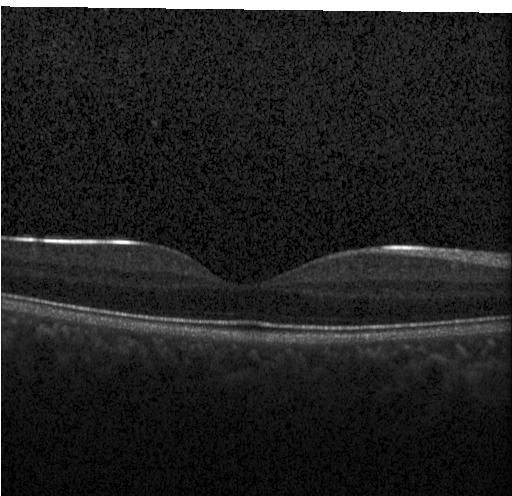

Impression: neither CNV, DME, nor drusen.